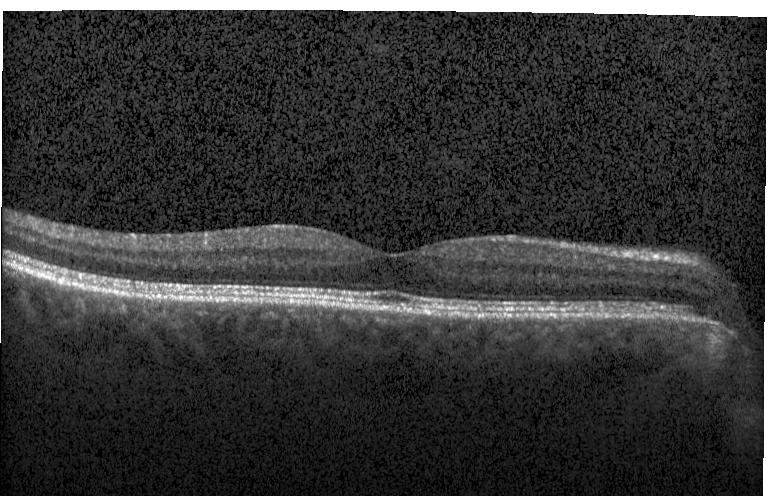

Impression: no evidence of choroidal neovascularization, diabetic macular edema, or drusen.